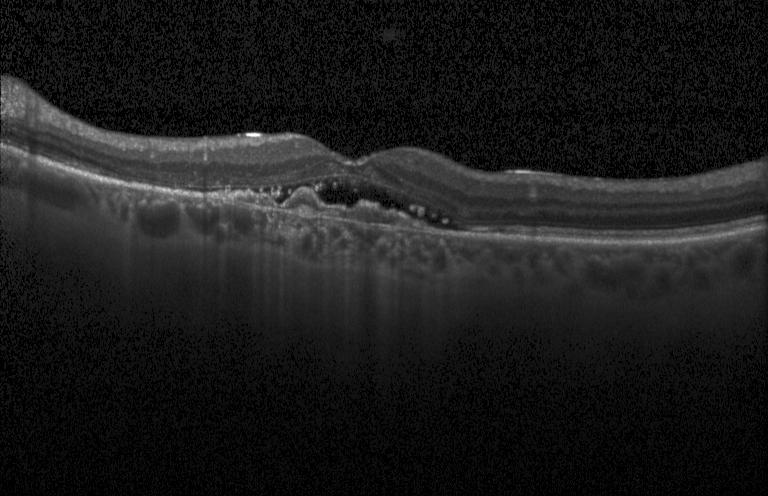
Finding: a choroidal neovascular membrane.